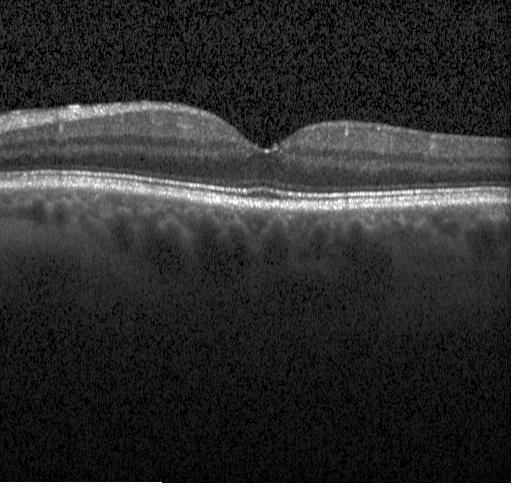 Diagnosis: no CNV, no DME, and no drusen.